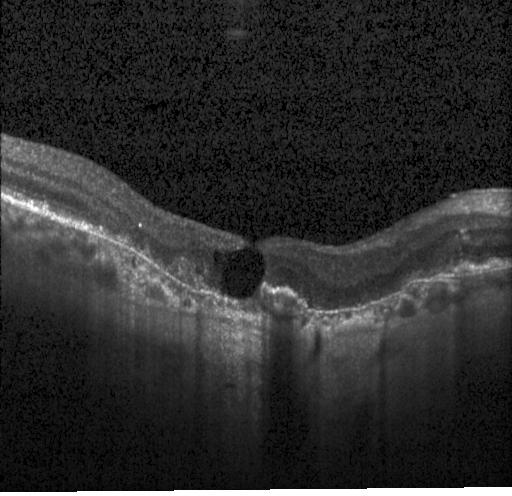

Macular OCT: CNV.